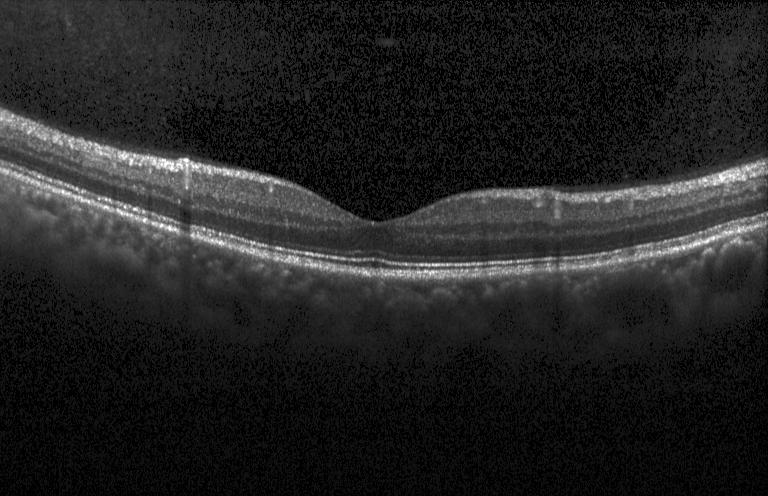 Retinal OCT cross-section. This B-scan demonstrates no choroidal neovascularization, no diabetic macular edema, and no drusen.